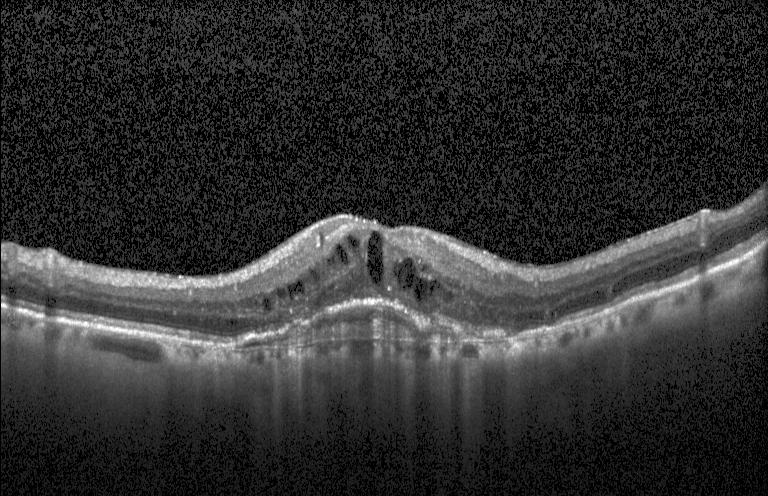

OCT finding: a choroidal neovascular membrane.